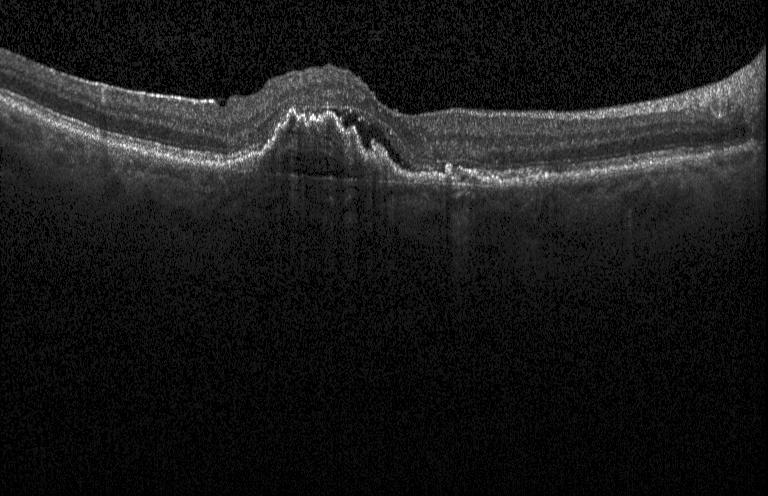
SD-OCT; retinal OCT B-scan.
Impression: choroidal neovascularization.